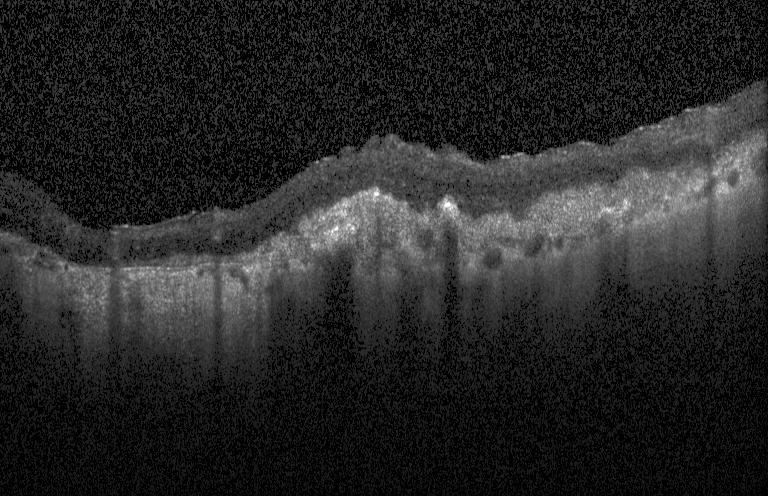
This B-scan demonstrates CNV.